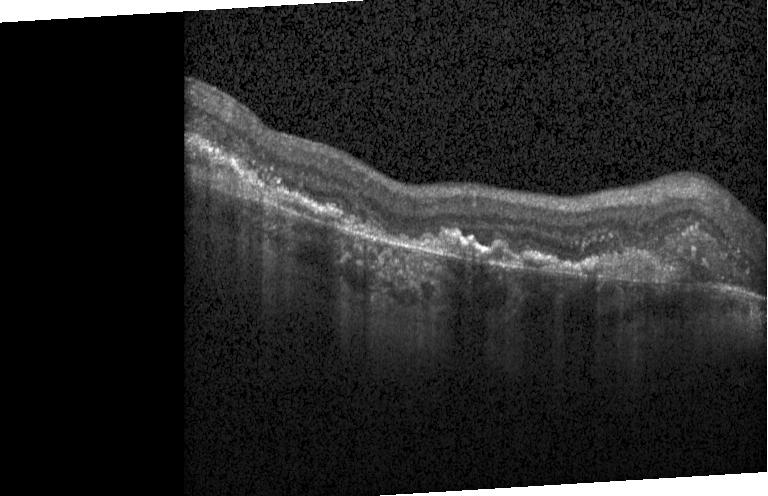

Diagnosis: a choroidal neovascular membrane.